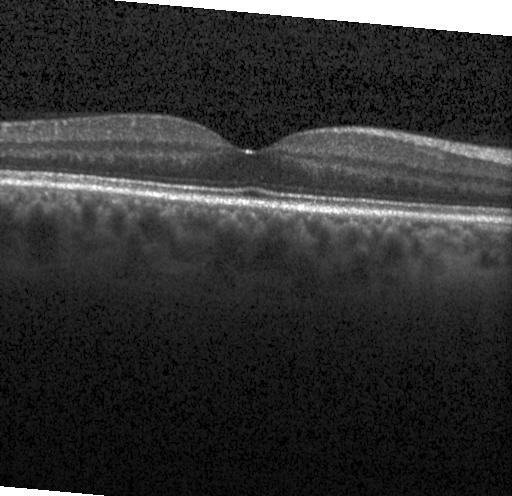

Diagnosis: no CNV, no DME, and no drusen.